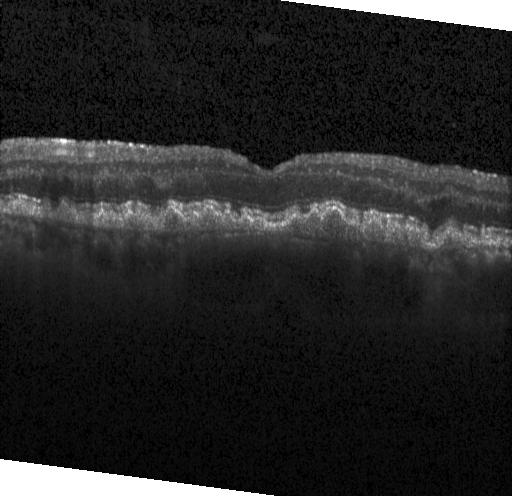

OCT line scan.
The scan shows choroidal neovascularization.